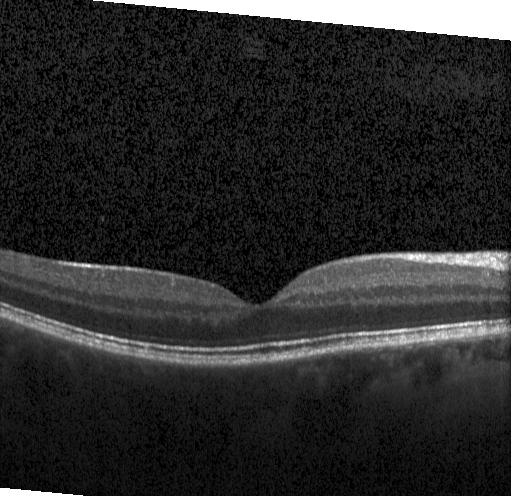 Dx: no choroidal neovascularization, diabetic macular edema, or drusen.